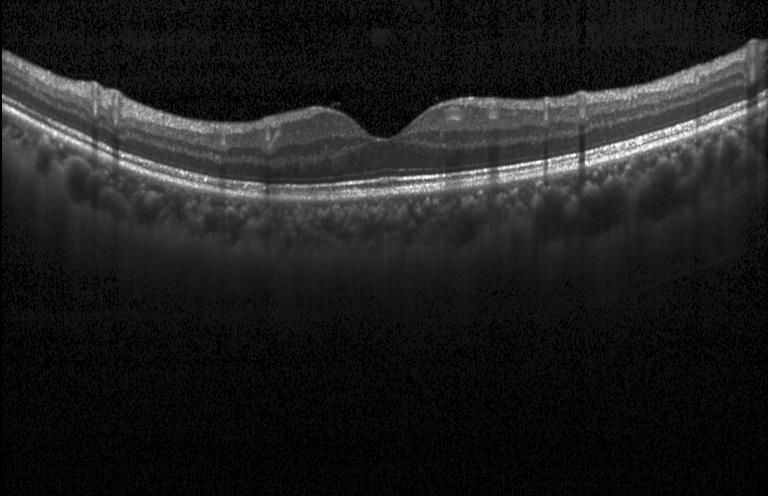

Diagnosis: no evidence of CNV, DME, or drusen.